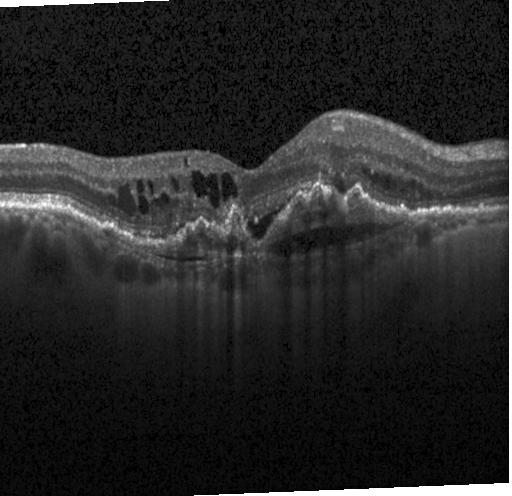
OCT scan showing CNV.